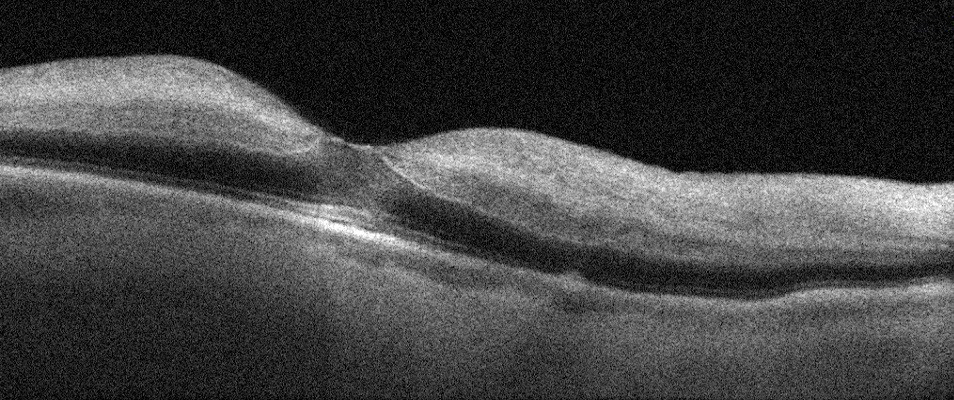

OCT B-scan. Finding: RAO.